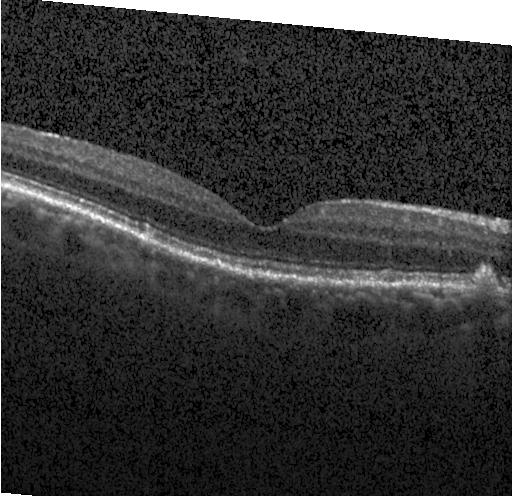 SD-OCT. Centered on the fovea. Retinal OCT cross-section — Macular OCT: multiple drusen.